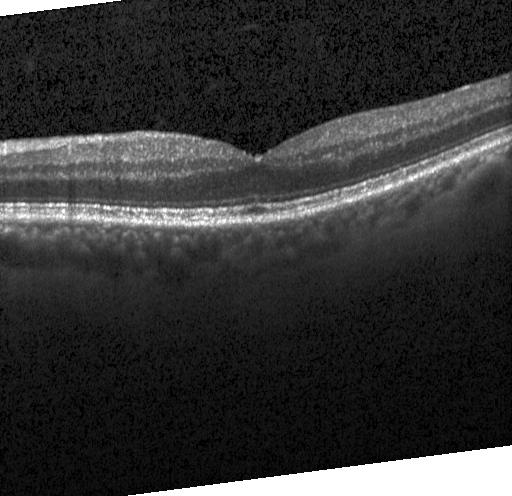 Optical coherence tomography B-scan. Heidelberg Spectralis OCT system. This B-scan demonstrates no choroidal neovascularization, diabetic macular edema, or drusen.